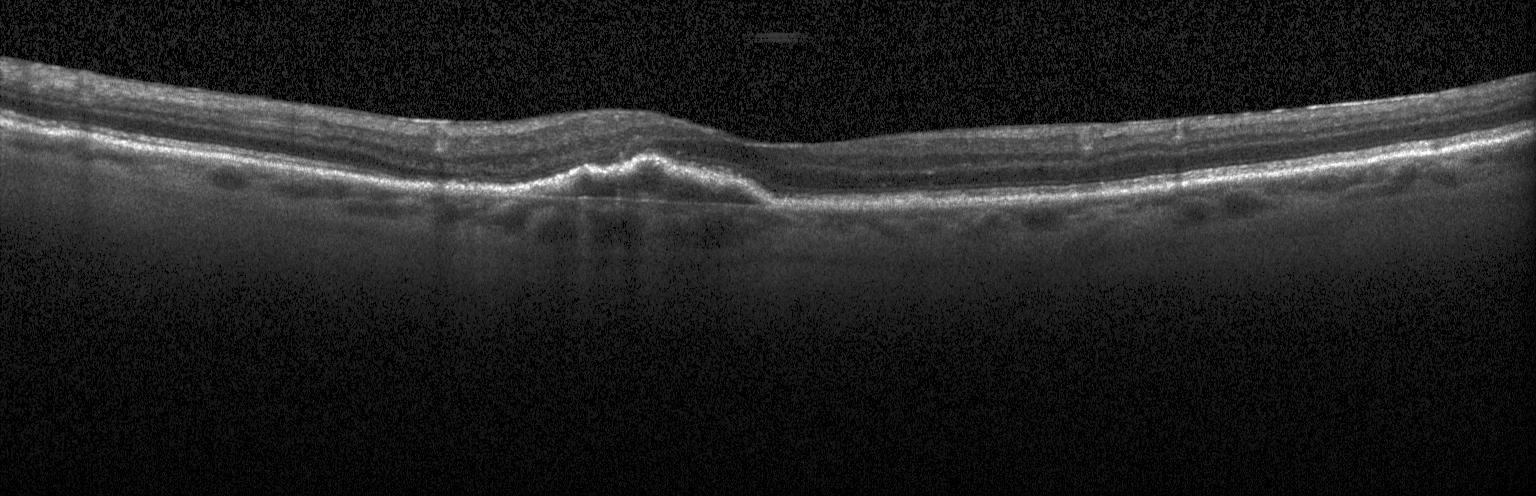 Optical coherence tomography scan. Dx: CNV.